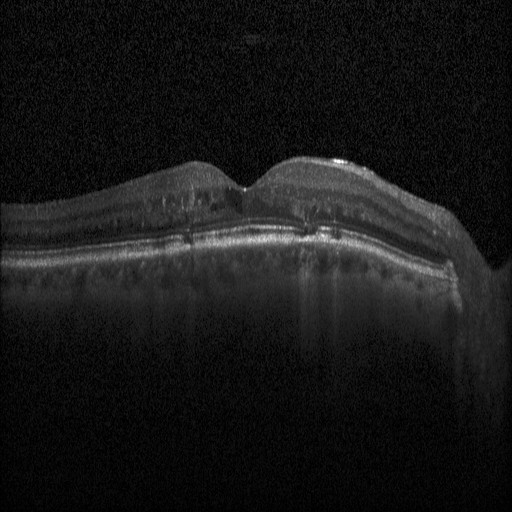 OCT B-scan; macular scan — Assessment: diabetic macular edema (DME).